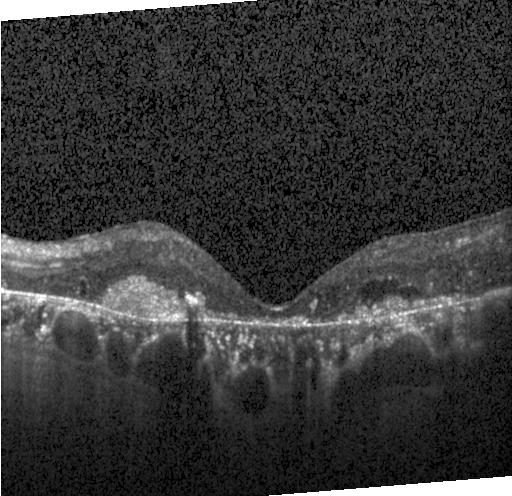

Through the macula, retinal OCT cross-section, spectral-domain OCT — This B-scan demonstrates a choroidal neovascular membrane.